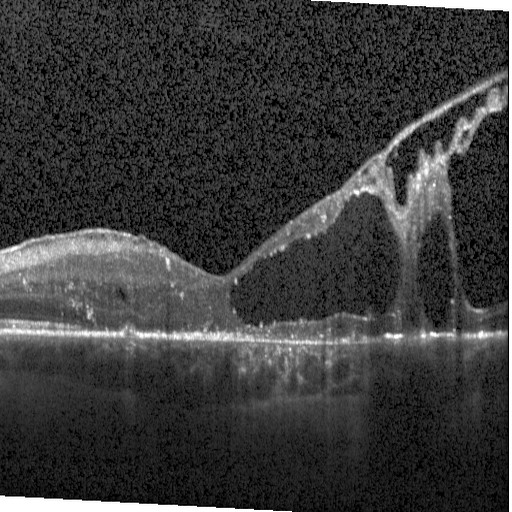 SD-OCT; Heidelberg Spectralis; OCT line scan; macular scan — Impression: diabetic macular edema (DME).